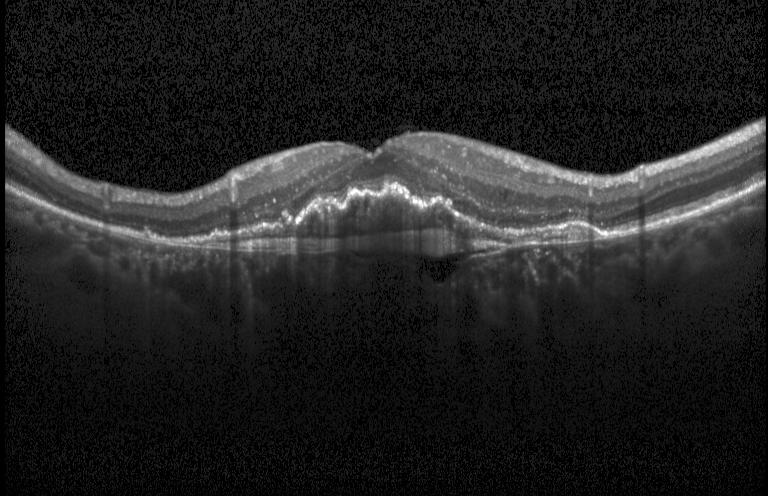 Finding: a choroidal neovascular membrane.